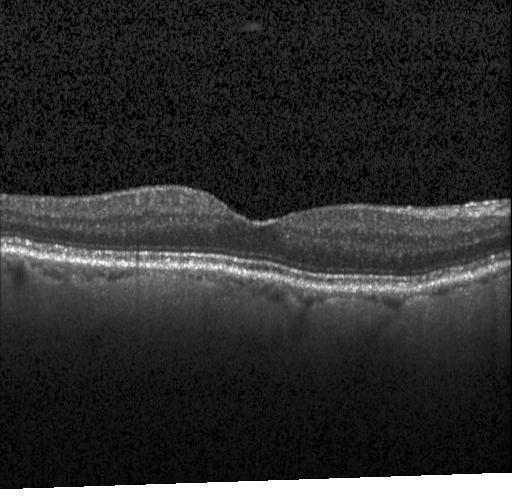

Macular scan, optical coherence tomography B-scan, spectral-domain optical coherence tomography, instrument: Heidelberg Spectralis. Macular OCT: no choroidal neovascularization, no diabetic macular edema, and no drusen.